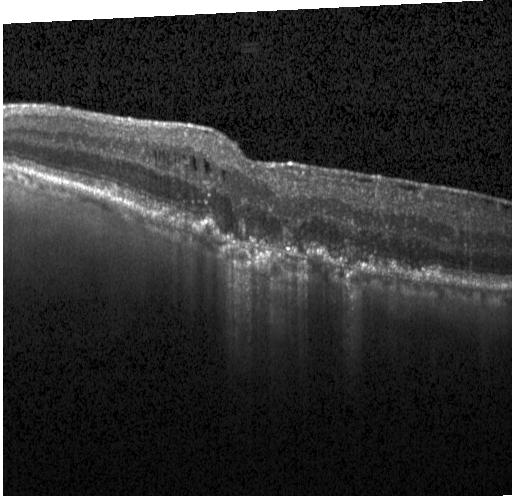
Retinal OCT B-scan · horizontal scan through the fovea · instrument: Heidelberg Spectralis
Diagnosis: choroidal neovascularization.